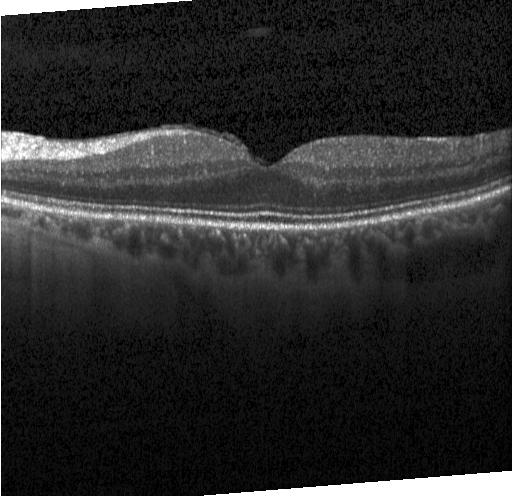
OCT line scan; macular scan.
Dx: no choroidal neovascularization, diabetic macular edema, or drusen.